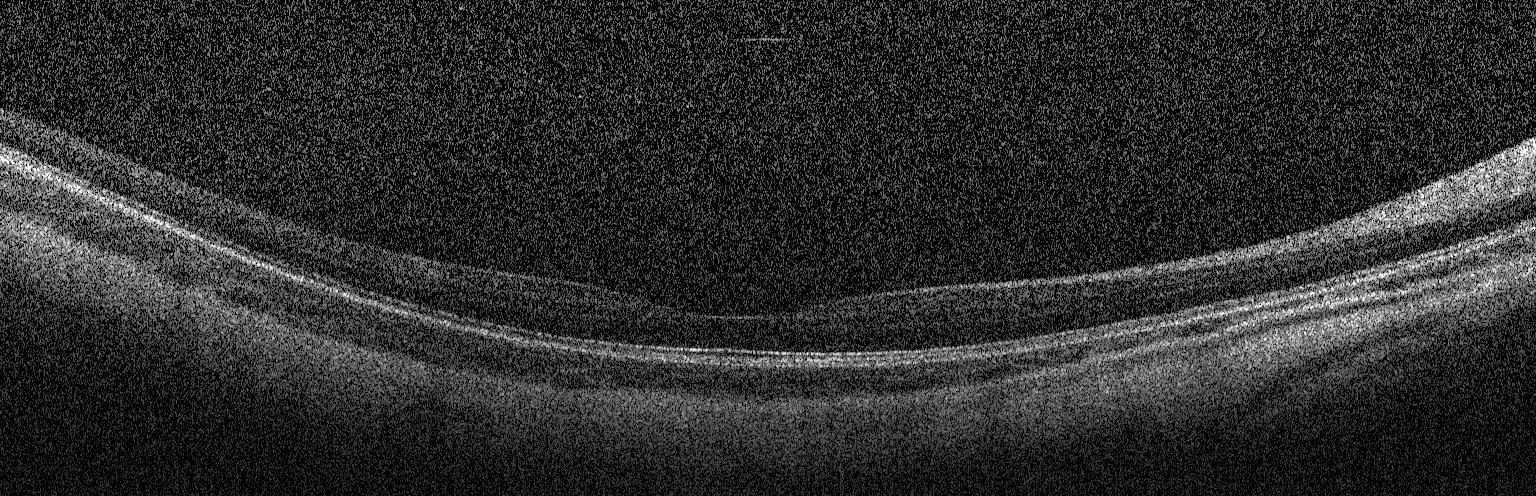

Diagnosis: neither CNV, DME, nor drusen.